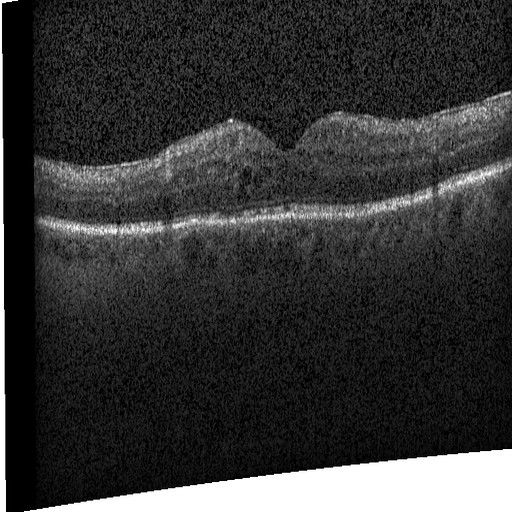
Optical coherence tomography B-scan, spectral-domain optical coherence tomography, horizontal scan through the fovea, acquired on a Heidelberg Spectralis — The scan shows diabetic macular edema.